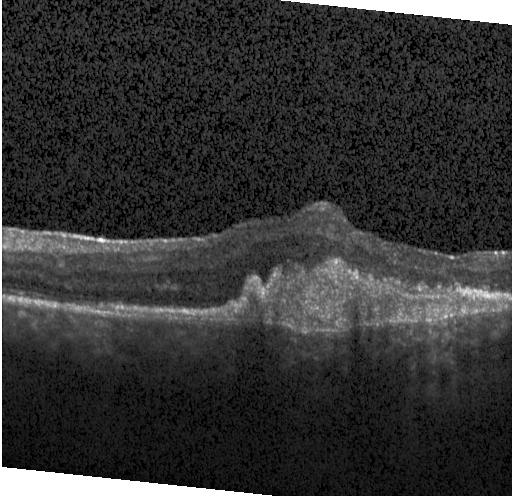

A choroidal neovascular membrane.